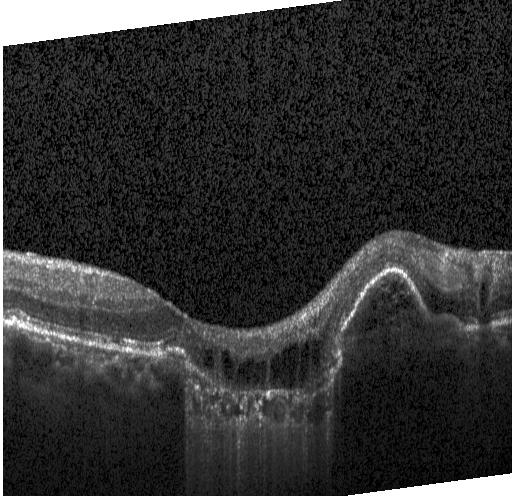 Retinal OCT cross-section; fovea-centered; instrument: Heidelberg Spectralis. This B-scan demonstrates a choroidal neovascular membrane.